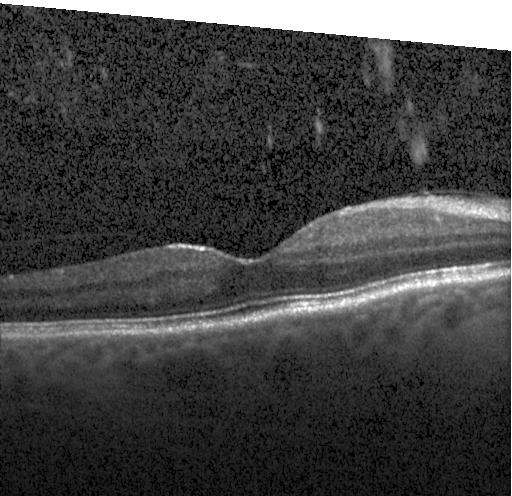

SD-OCT; optical coherence tomography scan; Heidelberg Spectralis OCT system. Macular OCT: no choroidal neovascularization, diabetic macular edema, or drusen.